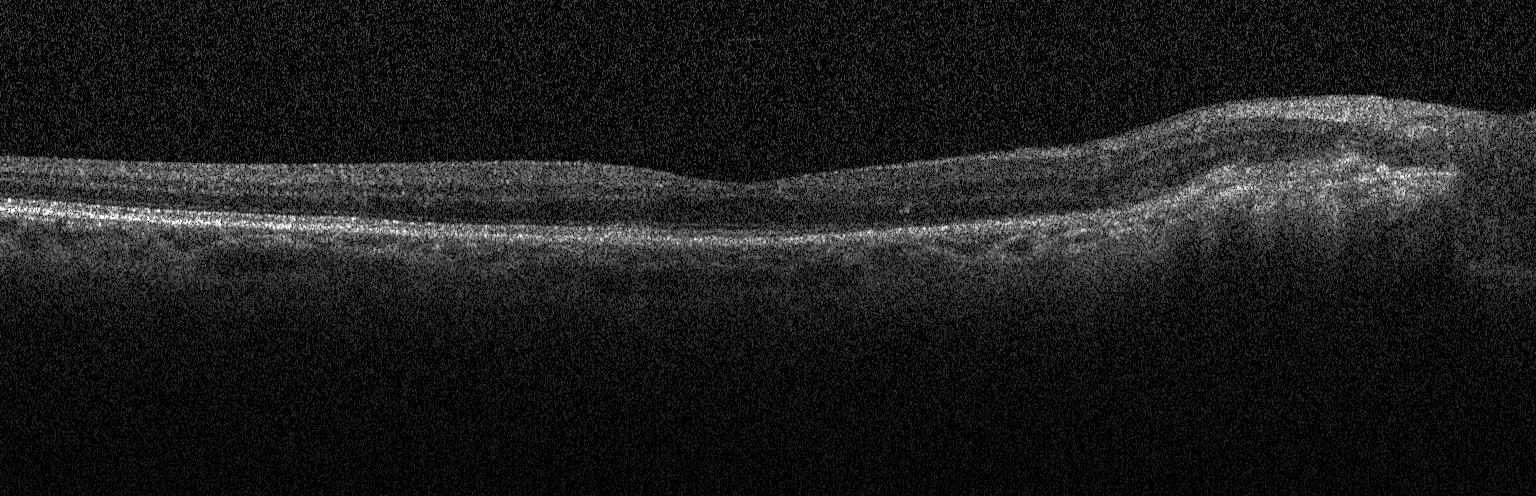
Spectral-domain optical coherence tomography, Heidelberg Spectralis OCT system, horizontal scan through the fovea, OCT line scan — A choroidal neovascular membrane.